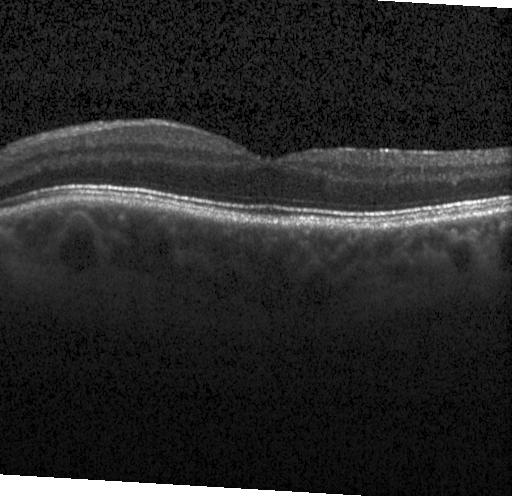 Diagnosis: no CNV, no DME, and no drusen.